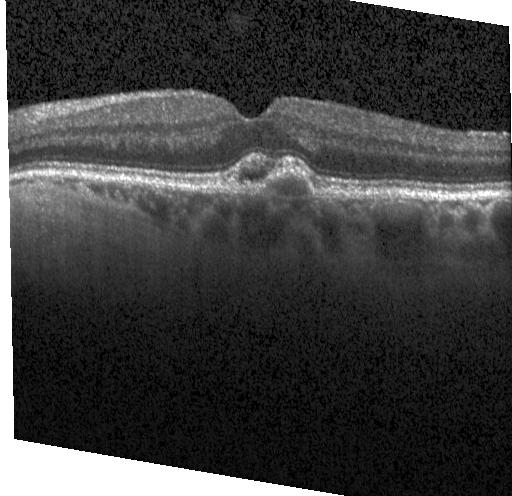

Through the macula. Optical coherence tomography B-scan. SD-OCT.
Diagnosis: a choroidal neovascular membrane.